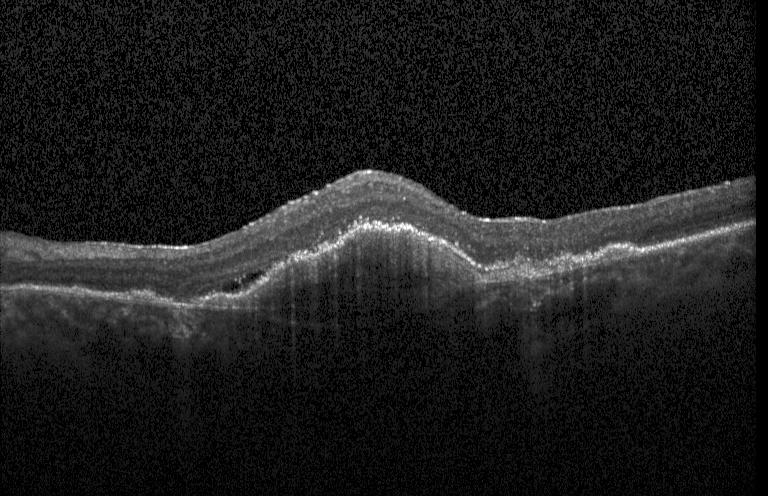

Impression: a choroidal neovascular membrane.